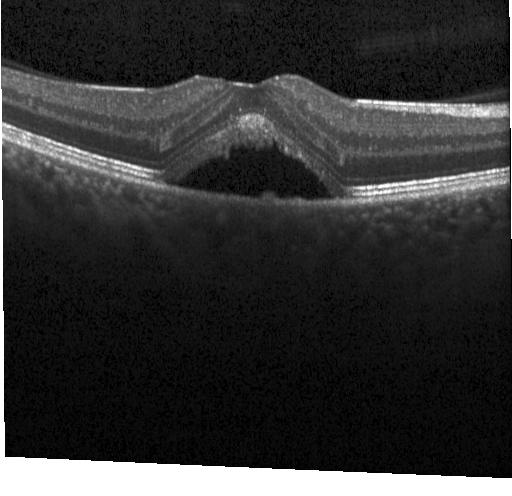 Retinal OCT B-scan · Heidelberg Spectralis · macular scan. A choroidal neovascular membrane.